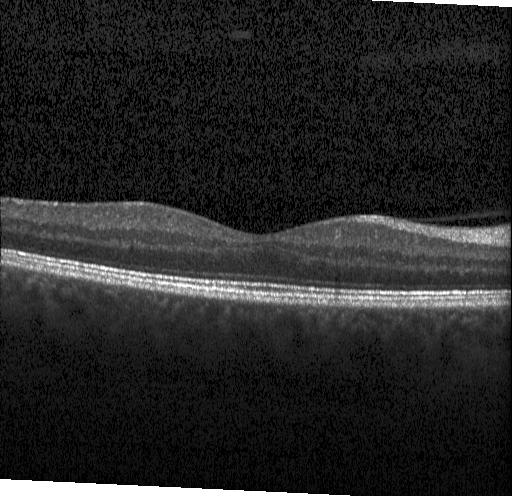

Spectral-domain OCT, retinal OCT B-scan, Heidelberg Spectralis, macular scan — Diagnosis: no choroidal neovascularization, diabetic macular edema, or drusen.